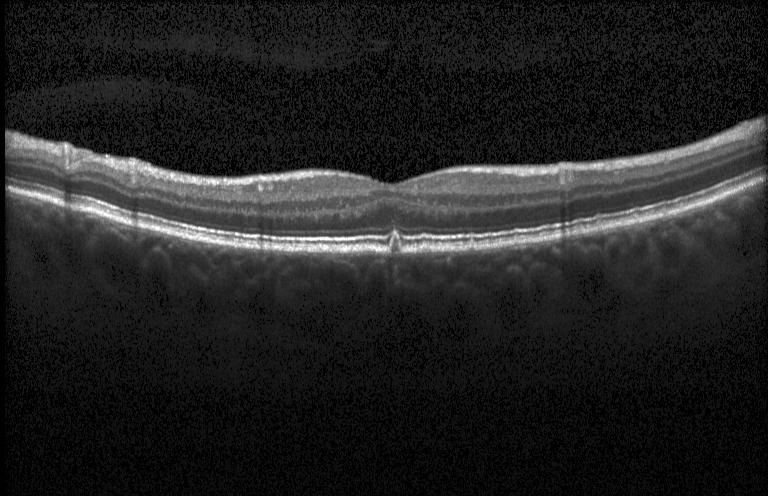
OCT B-scan showing sub-RPE drusenoid deposits.